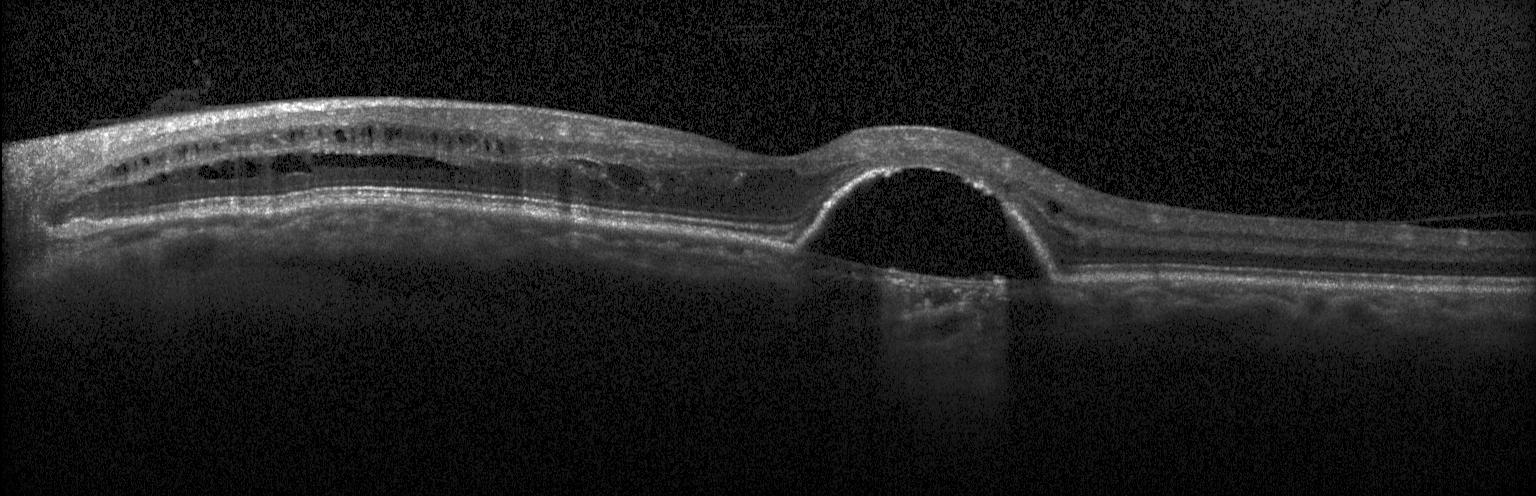

Optical coherence tomography B-scan; horizontal scan through the fovea; spectral-domain OCT — This B-scan demonstrates a choroidal neovascular membrane.